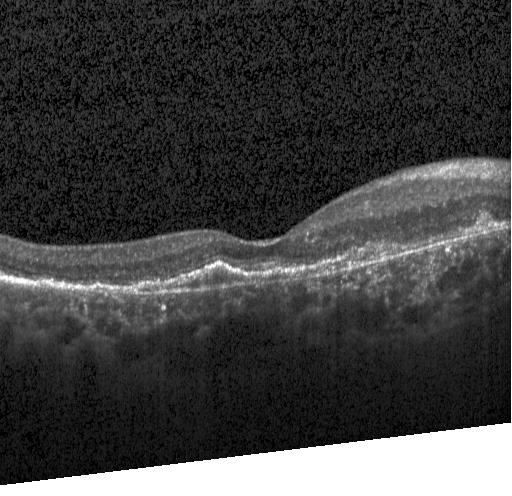

Spectral-domain OCT, acquired on a Heidelberg Spectralis, retinal OCT B-scan, horizontal scan through the fovea. Diagnosis: a choroidal neovascular membrane.